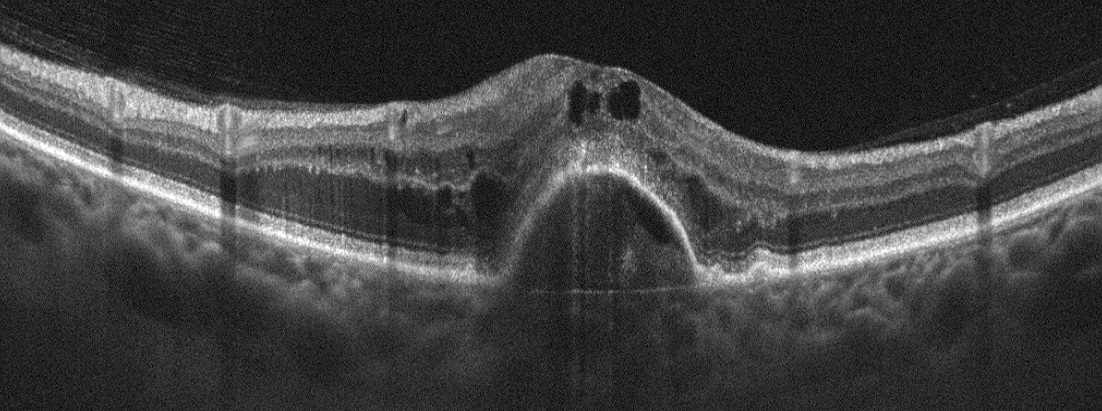 OCT scan showing AMD.